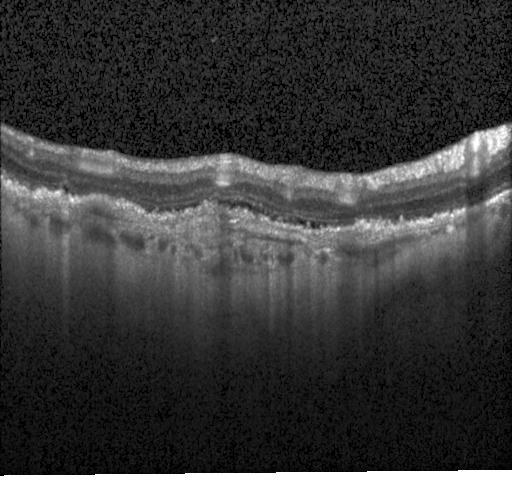 This B-scan demonstrates CNV.